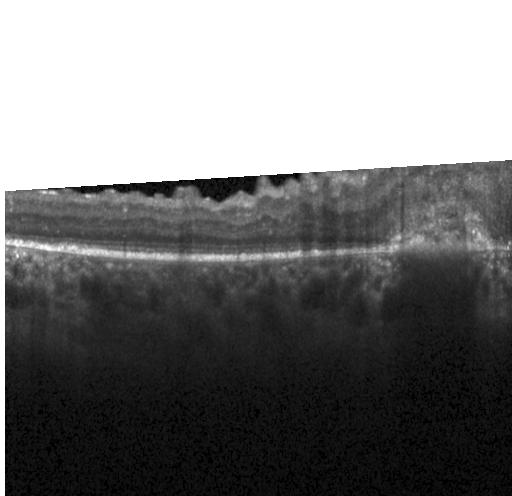
Dx: choroidal neovascularization.